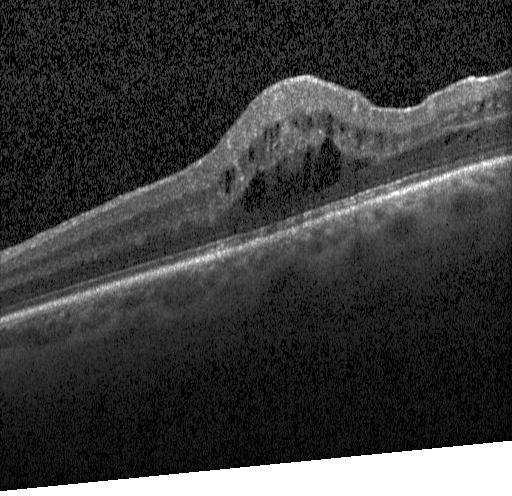 Horizontal scan through the fovea, retinal OCT B-scan, Heidelberg Spectralis OCT system. OCT finding: DME.